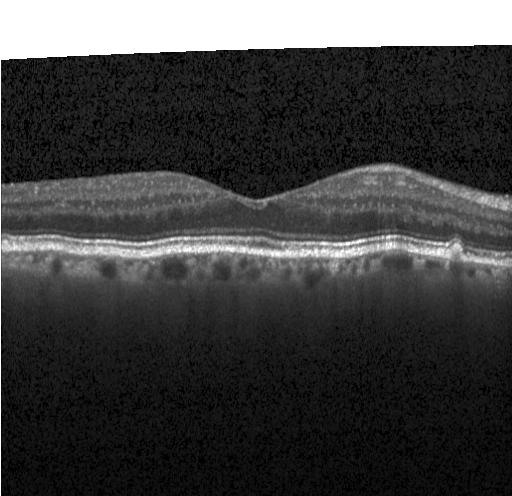 OCT B-scan. Diagnosis: neither choroidal neovascularization, diabetic macular edema, nor drusen.